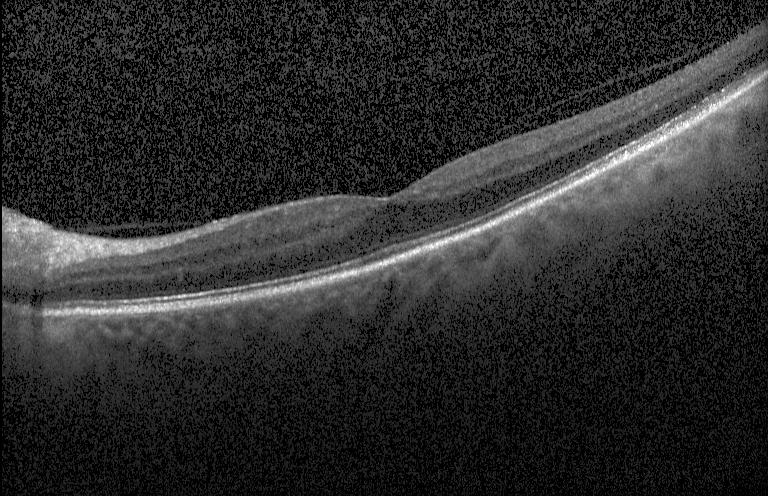
Macular scan; retinal OCT cross-section. Assessment: neither CNV, DME, nor drusen.